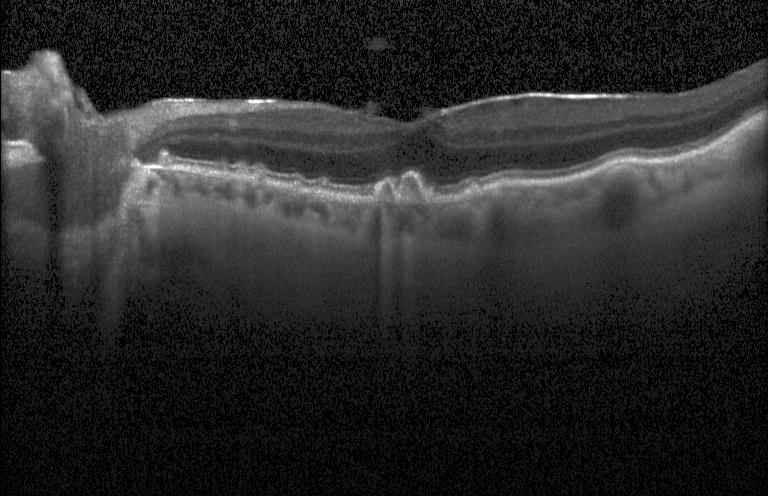 The scan shows drusen.